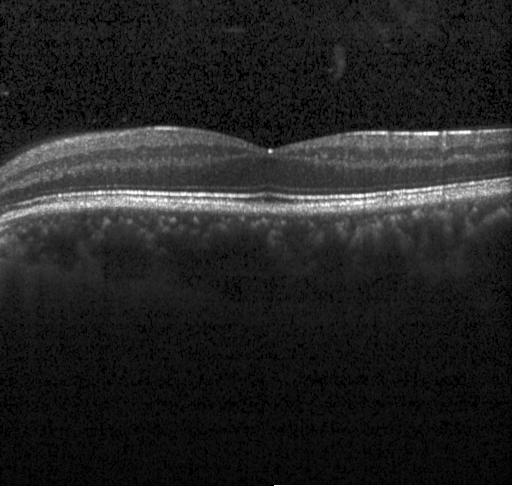 SD-OCT, retinal OCT B-scan
OCT finding: no evidence of CNV, DME, or drusen.